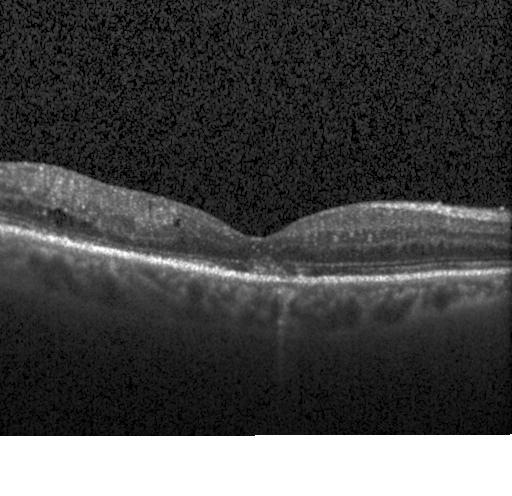 Retinal OCT cross-section, Heidelberg Spectralis.
Assessment: DME.